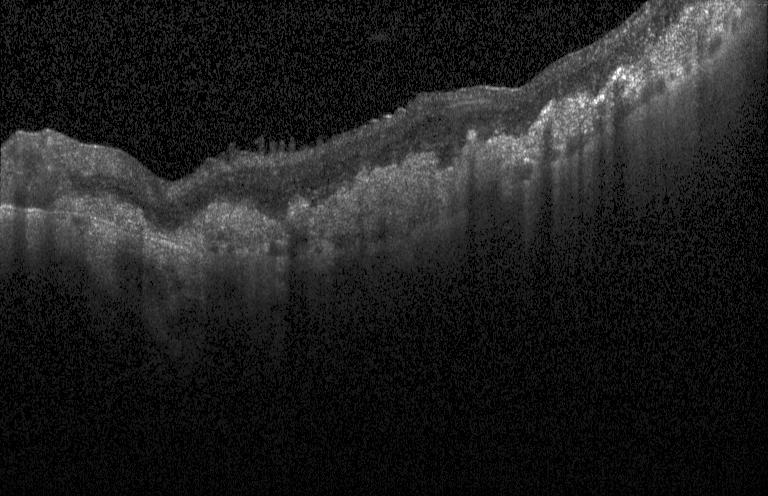
OCT line scan. Diagnosis: a choroidal neovascular membrane.